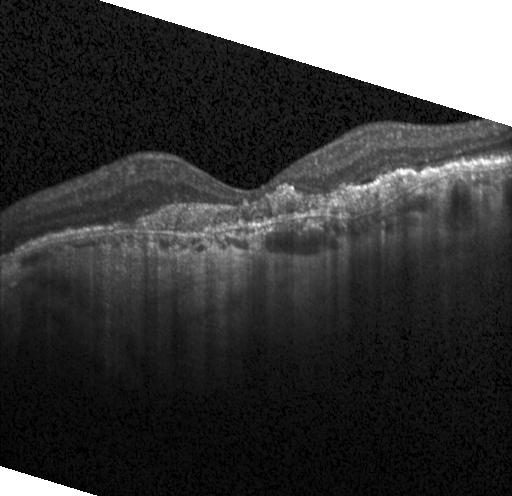 This B-scan demonstrates a choroidal neovascular membrane.